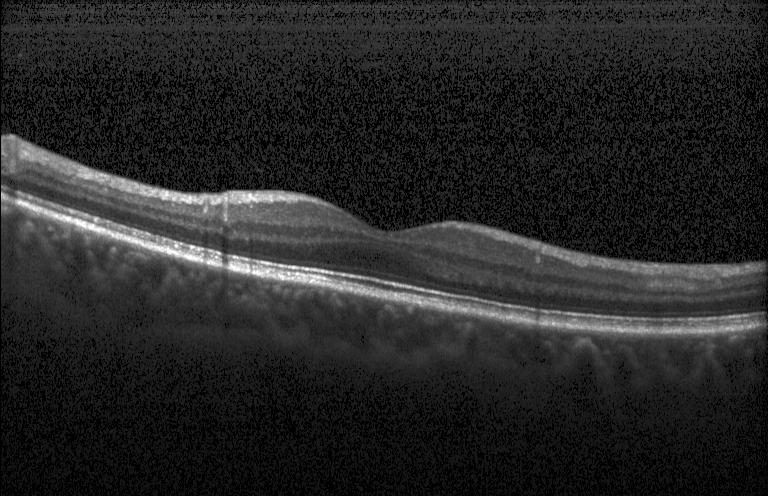 Retinal OCT cross-section showing no choroidal neovascularization, diabetic macular edema, or drusen.